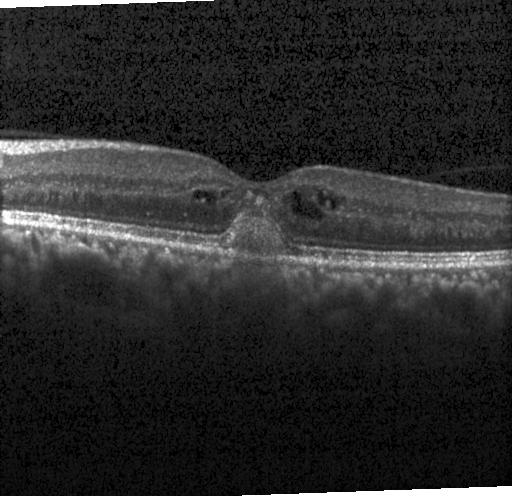

OCT line scan.
OCT finding: a choroidal neovascular membrane.